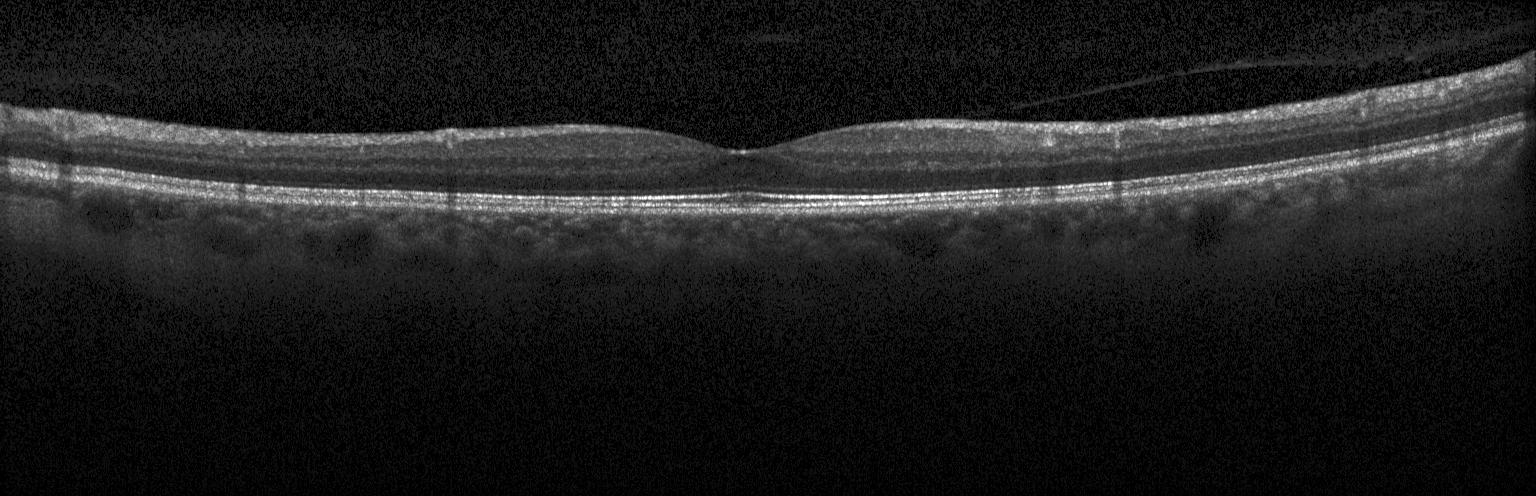 Retinal OCT cross-section.
Impression: no choroidal neovascularization, diabetic macular edema, or drusen.